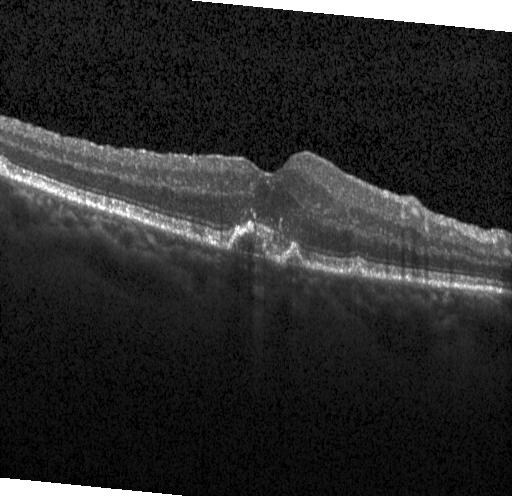 OCT finding: sub-RPE drusenoid deposits.